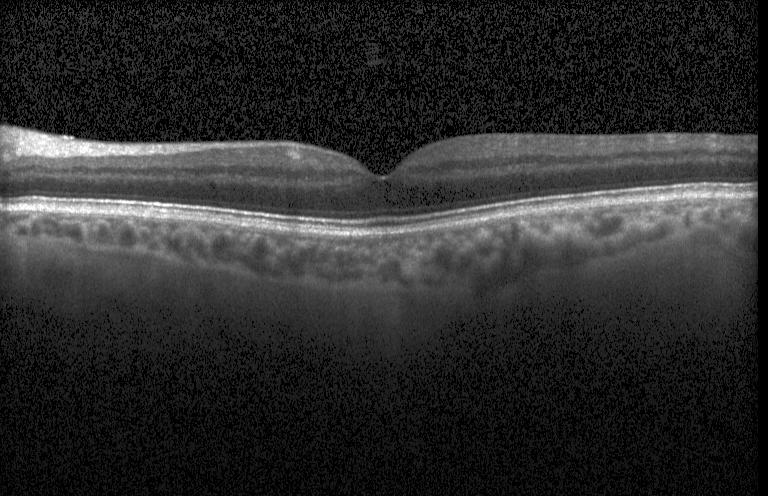

Finding: neither CNV, DME, nor drusen.